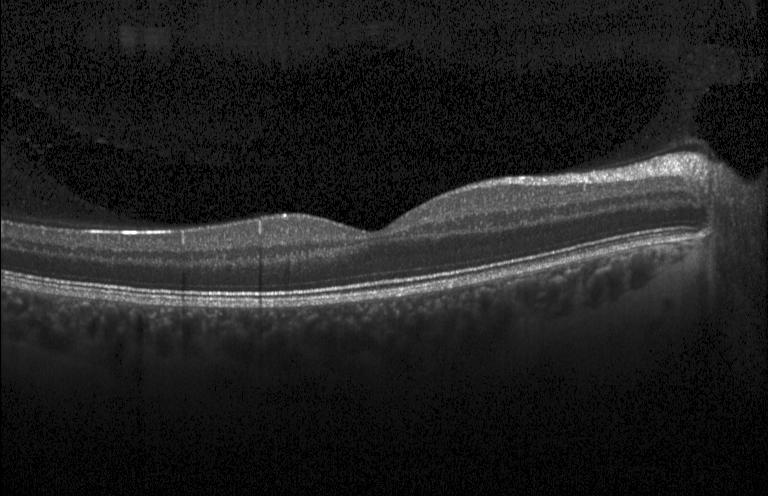 Macular OCT: neither choroidal neovascularization, diabetic macular edema, nor drusen.